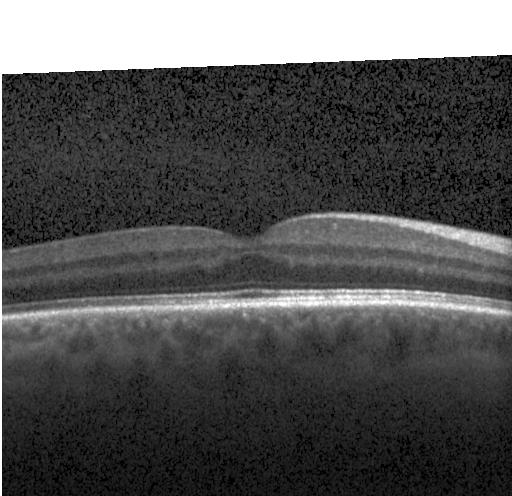 Spectral-domain OCT B-scan: no choroidal neovascularization, diabetic macular edema, or drusen.